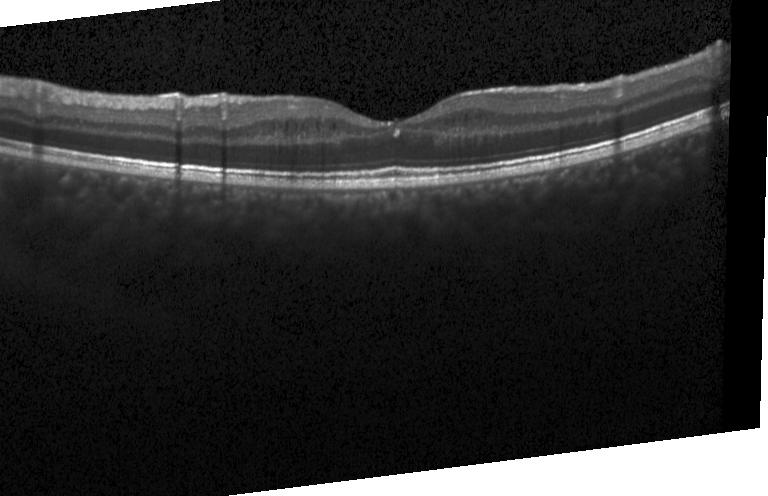
Optical coherence tomography scan; Heidelberg Spectralis — Finding: DME.